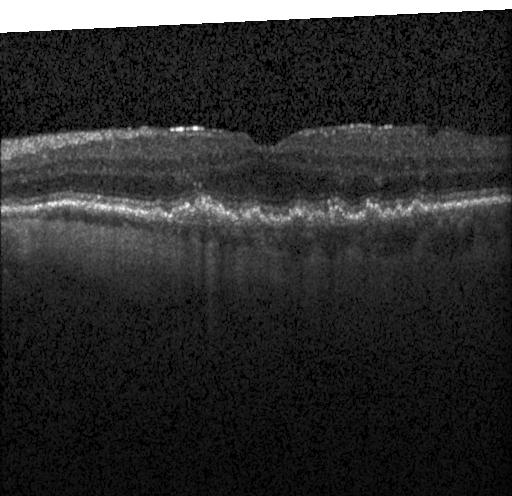 Fovea-centered; optical coherence tomography scan; acquired on a Heidelberg Spectralis; spectral-domain OCT — OCT finding: multiple drusen.